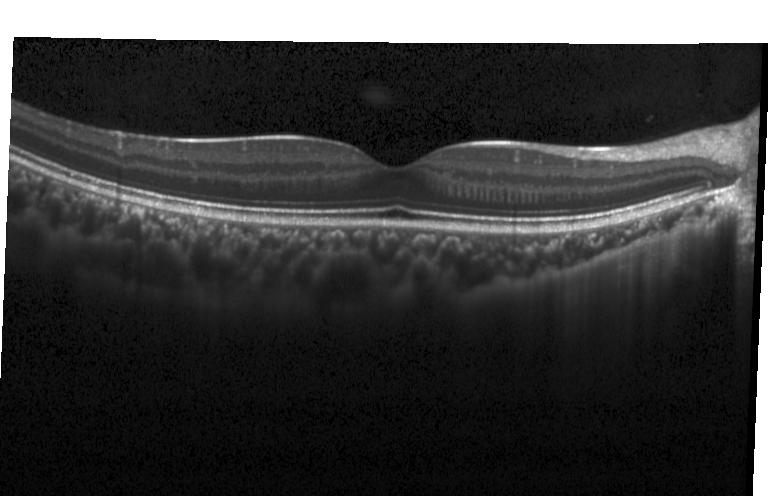
Finding: neither choroidal neovascularization, diabetic macular edema, nor drusen.